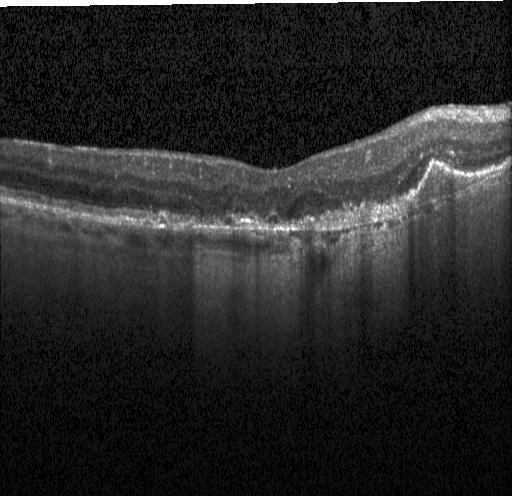

SD-OCT; OCT B-scan; instrument: Heidelberg Spectralis.
Dx: CNV.